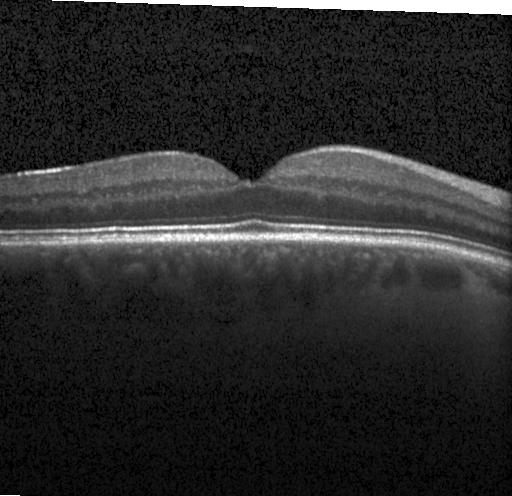

Centered on the fovea · spectral-domain OCT · Heidelberg Spectralis OCT system · optical coherence tomography B-scan. Diagnosis: neither choroidal neovascularization, diabetic macular edema, nor drusen.